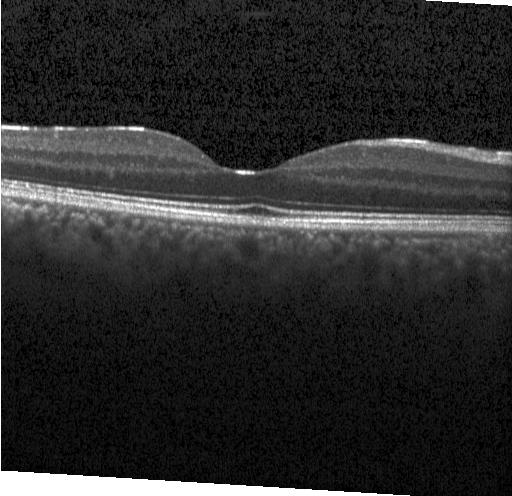 OCT line scan, Heidelberg Spectralis, fovea-centered.
Impression: no evidence of CNV, DME, or drusen.